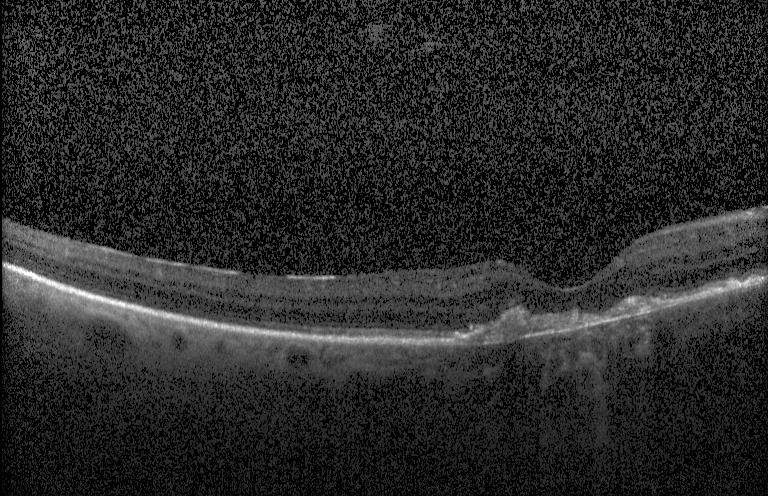
Optical coherence tomography scan · through the macula
The scan shows a choroidal neovascular membrane.